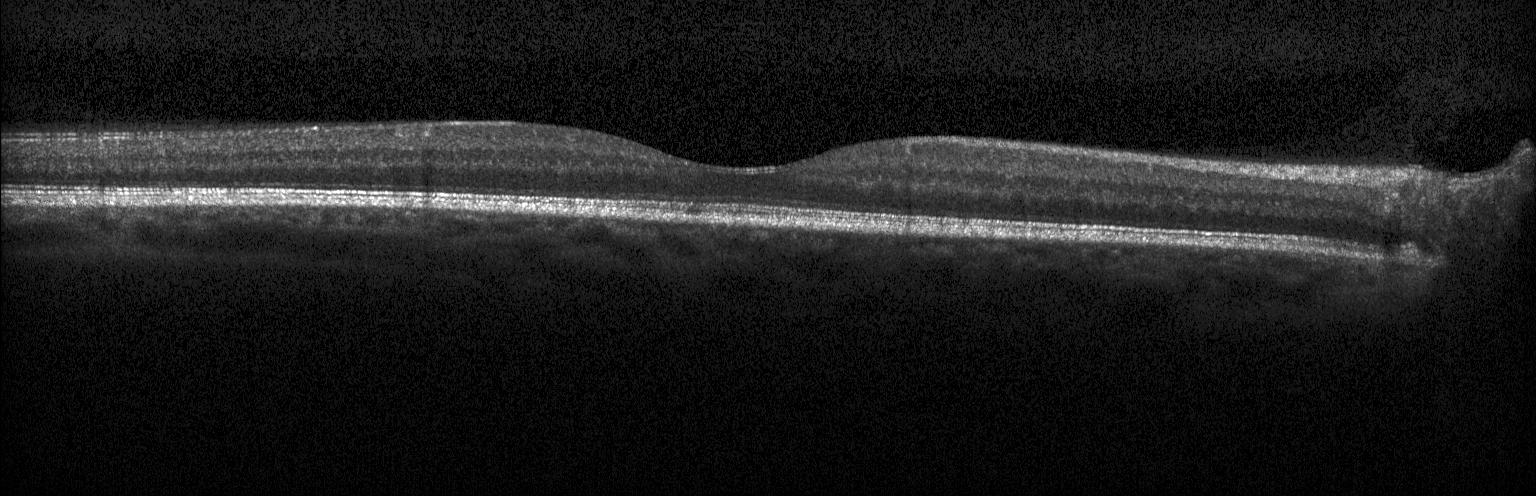

Horizontal scan through the fovea. Spectral-domain optical coherence tomography. Acquired on a Heidelberg Spectralis. Retinal OCT cross-section. Dx: no CNV, no DME, and no drusen.